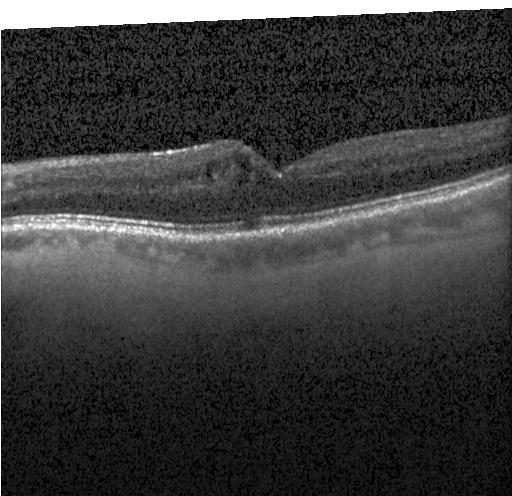 OCT B-scan showing diabetic macular edema.